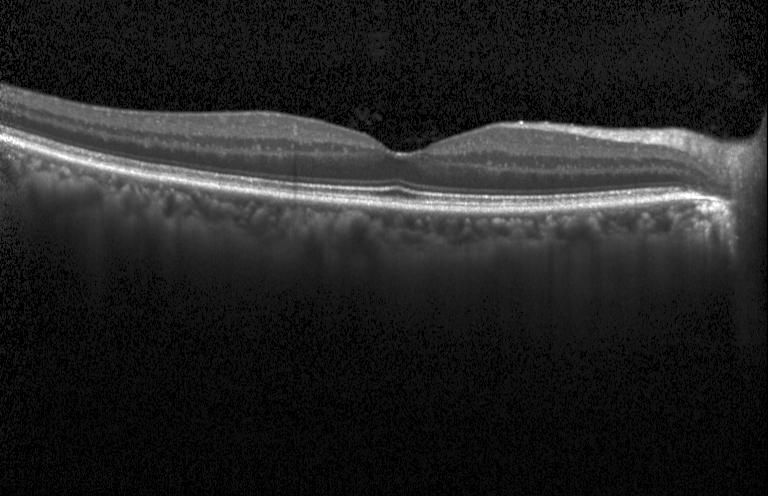

Heidelberg Spectralis OCT system; spectral-domain OCT; optical coherence tomography scan; macular scan. The scan shows no evidence of choroidal neovascularization, diabetic macular edema, or drusen.